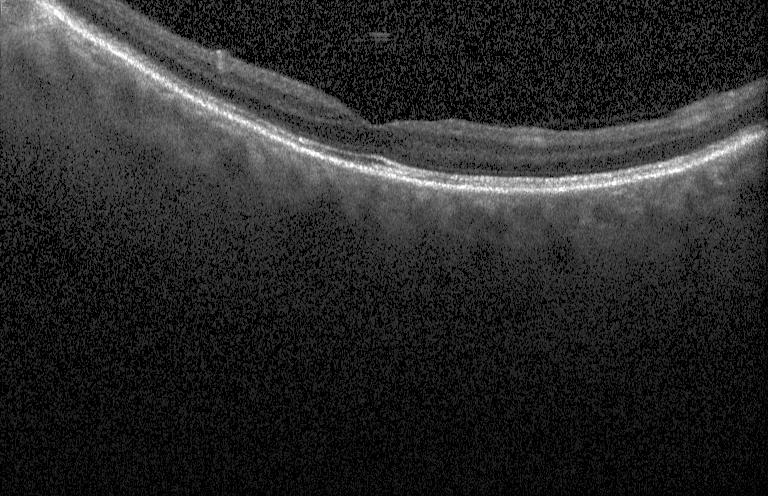
Retinal OCT cross-section; macular scan; Heidelberg Spectralis
Finding: neither CNV, DME, nor drusen.